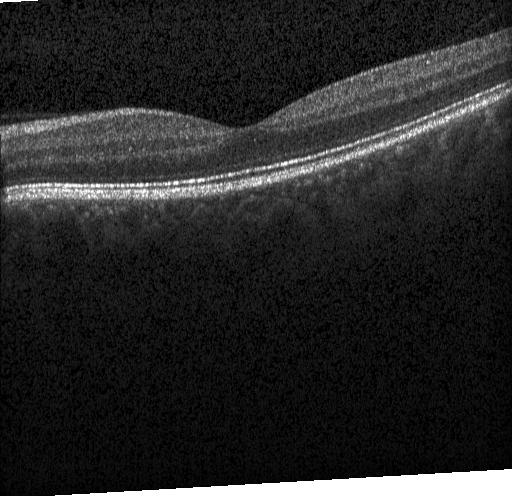

Heidelberg Spectralis OCT system. Retinal OCT cross-section
Diagnosis: neither choroidal neovascularization, diabetic macular edema, nor drusen.